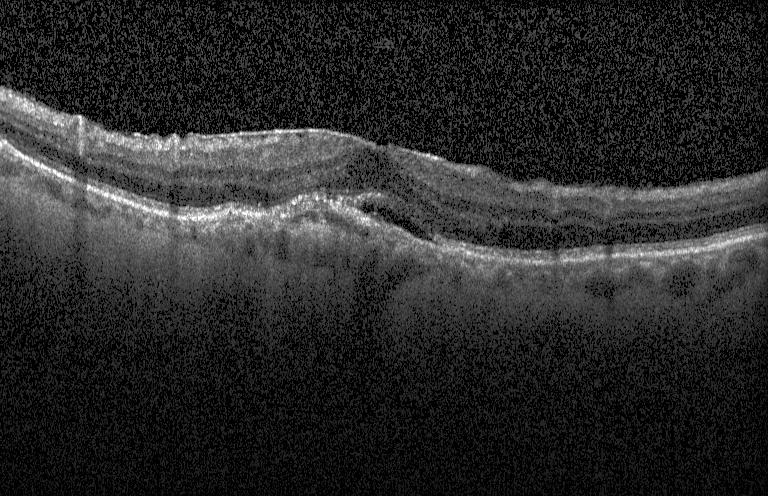
Retinal OCT cross-section. This B-scan demonstrates choroidal neovascularization (CNV).